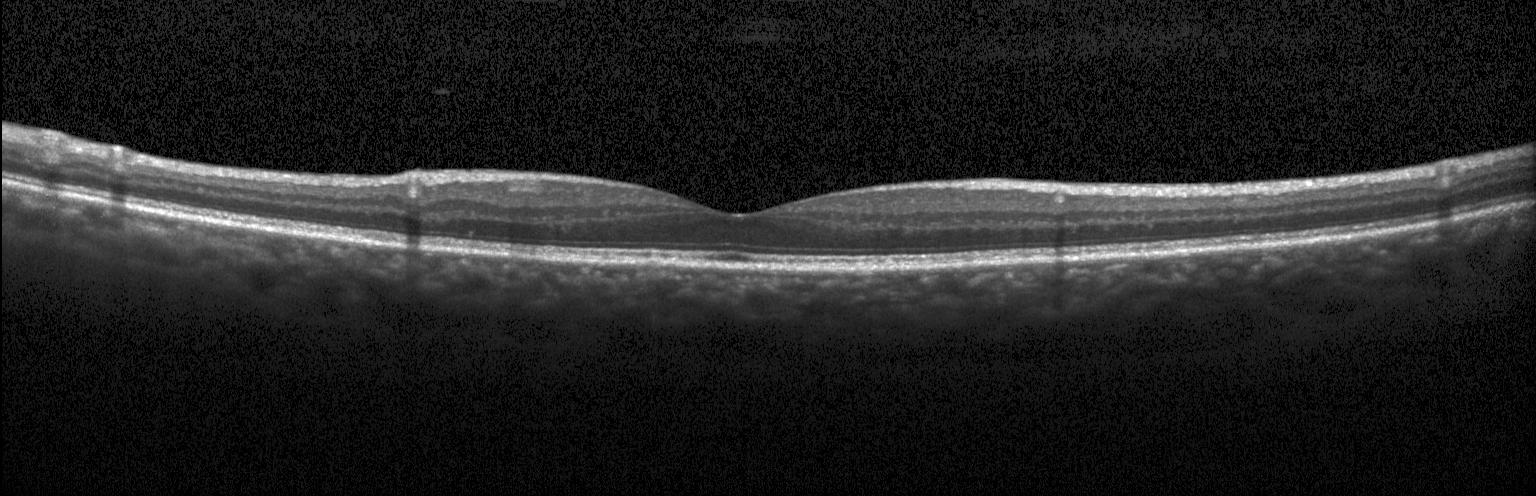
Retinal OCT cross-section · spectral-domain optical coherence tomography · fovea-centered · Heidelberg Spectralis
Diagnosis: neither choroidal neovascularization, diabetic macular edema, nor drusen.